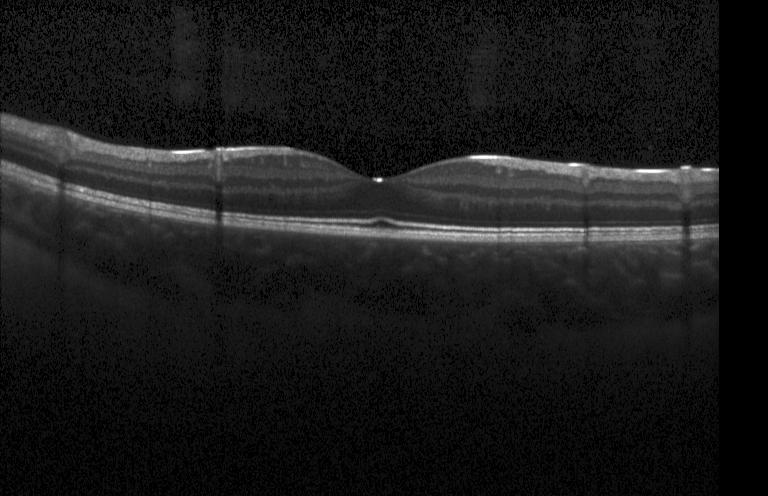

Macular OCT: neither choroidal neovascularization, diabetic macular edema, nor drusen.